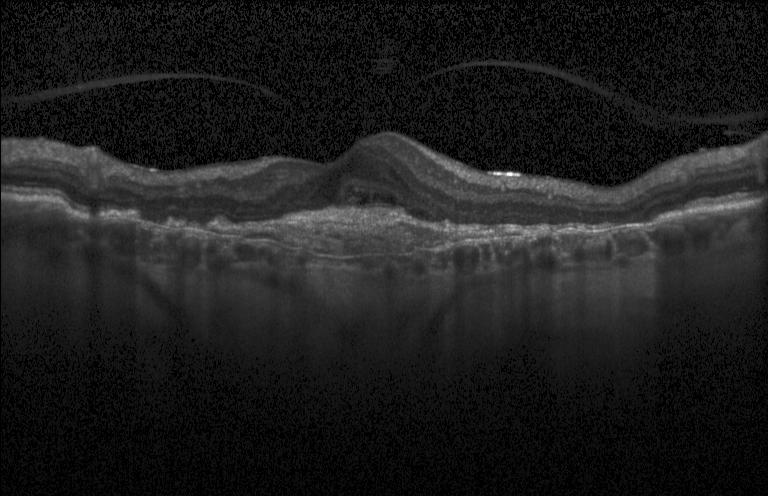
Fovea-centered. Instrument: Heidelberg Spectralis. OCT line scan. Diagnosis: choroidal neovascularization.